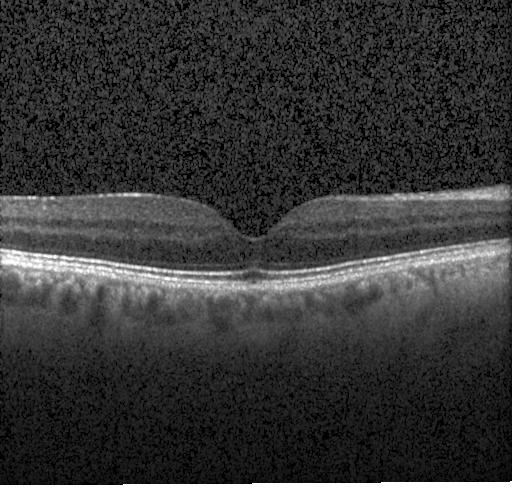 The scan shows neither choroidal neovascularization, diabetic macular edema, nor drusen.